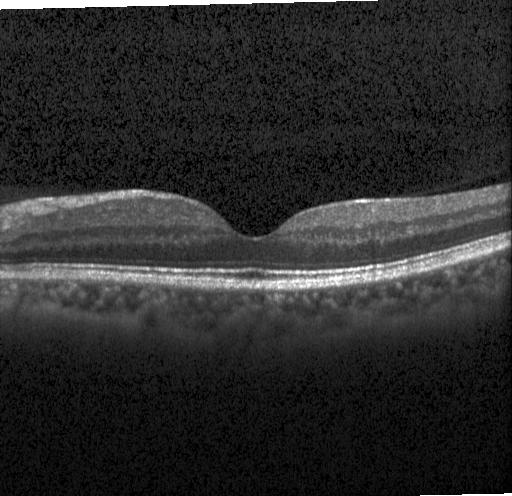
SD-OCT. Heidelberg Spectralis OCT system. Retinal OCT B-scan — Impression: neither choroidal neovascularization, diabetic macular edema, nor drusen.